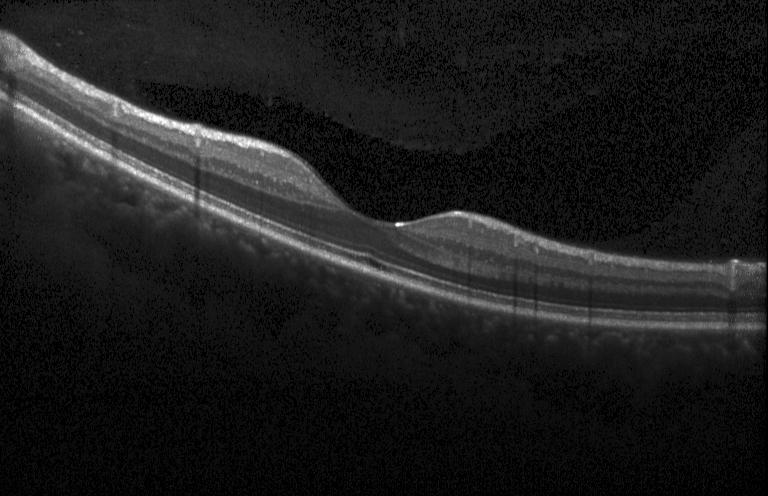

Optical coherence tomography B-scan — Finding: neither choroidal neovascularization, diabetic macular edema, nor drusen.